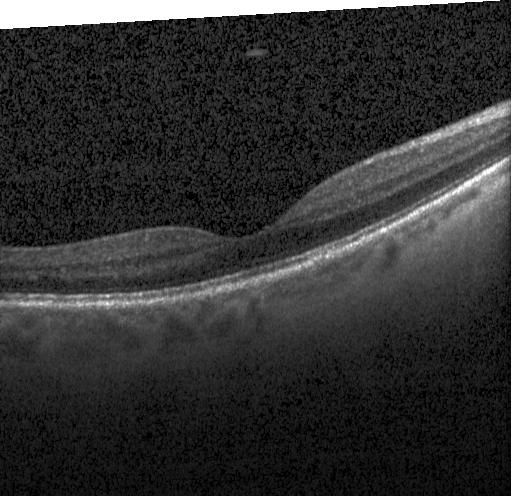

Diagnosis: no evidence of choroidal neovascularization, diabetic macular edema, or drusen.